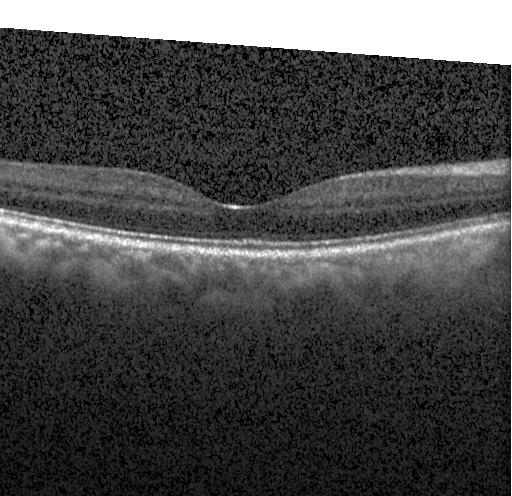

SD-OCT; retinal OCT cross-section; fovea-centered.
Finding: no evidence of choroidal neovascularization, diabetic macular edema, or drusen.